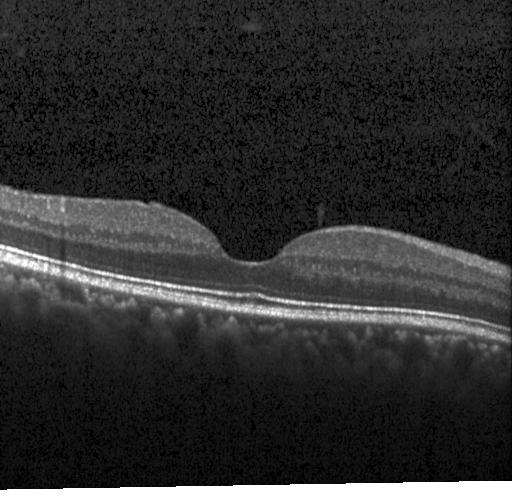 Heidelberg Spectralis OCT system. Spectral-domain OCT. Retinal OCT cross-section. Finding: no evidence of choroidal neovascularization, diabetic macular edema, or drusen.